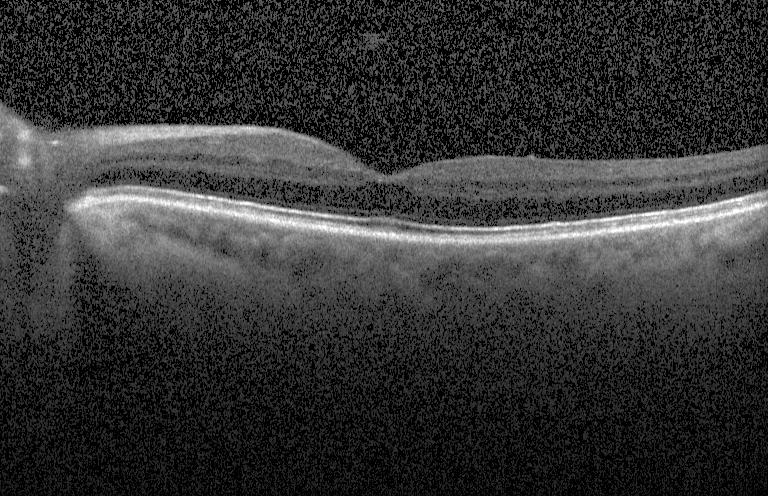
Retinal OCT B-scan; through the macula; spectral-domain optical coherence tomography; Heidelberg Spectralis OCT system
The scan shows no choroidal neovascularization, diabetic macular edema, or drusen.